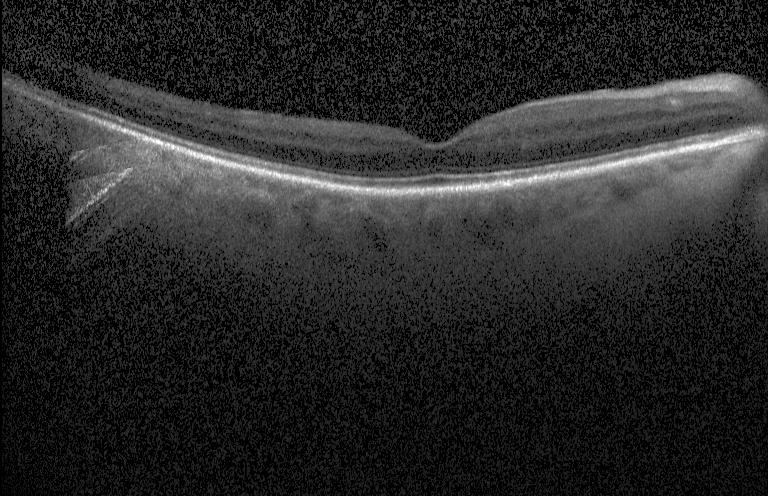

Dx: no evidence of CNV, DME, or drusen.